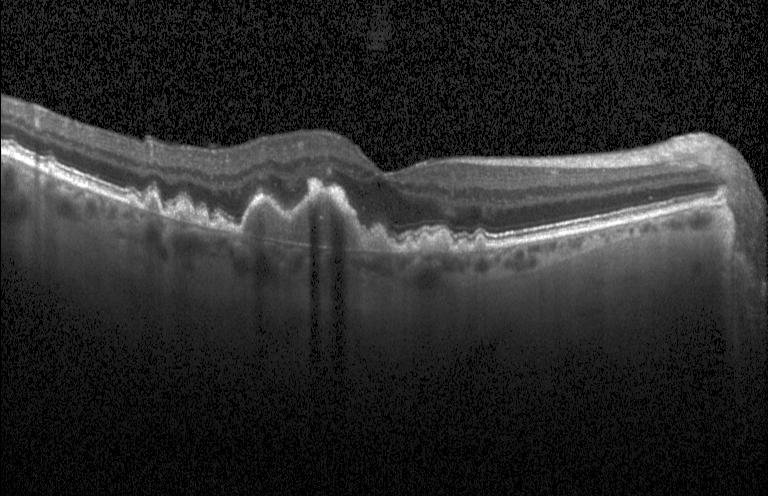 OCT line scan, Heidelberg Spectralis
Diagnosis: a choroidal neovascular membrane.